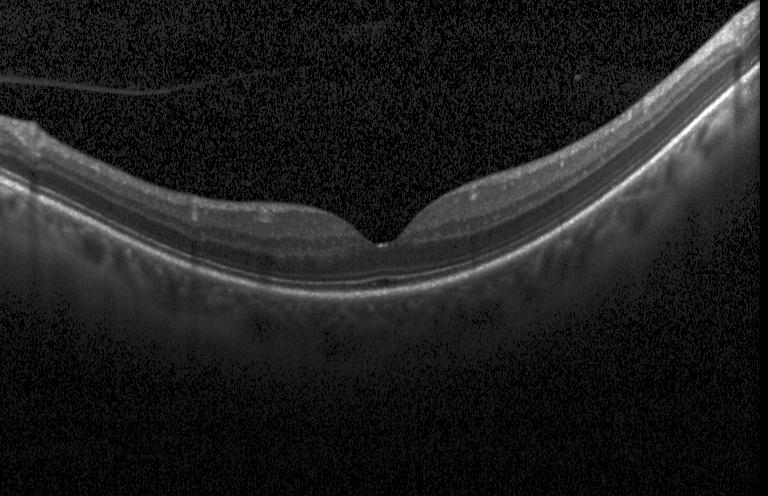 OCT finding: no choroidal neovascularization, diabetic macular edema, or drusen.